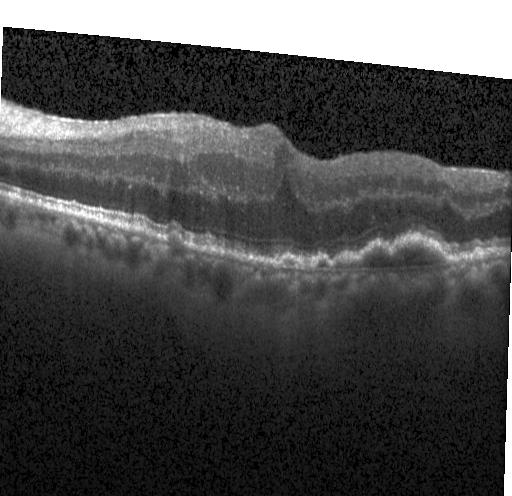 Retinal OCT cross-section
Impression: choroidal neovascularization (CNV).